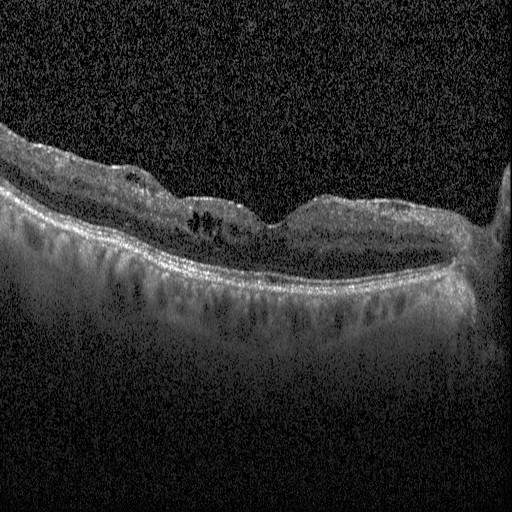

Instrument: Heidelberg Spectralis, optical coherence tomography B-scan, spectral-domain OCT.
Diabetic macular edema.